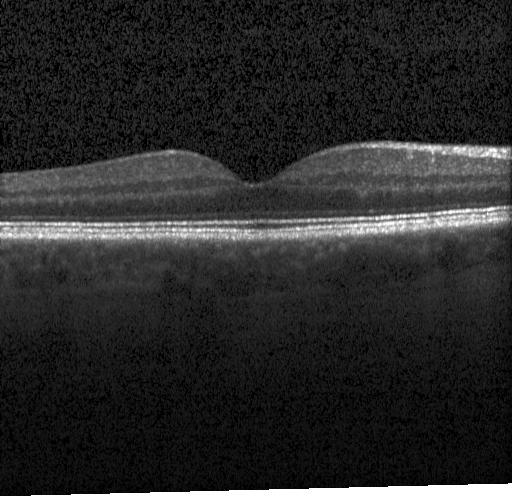
OCT B-scan; SD-OCT; centered on the fovea.
No choroidal neovascularization, diabetic macular edema, or drusen.